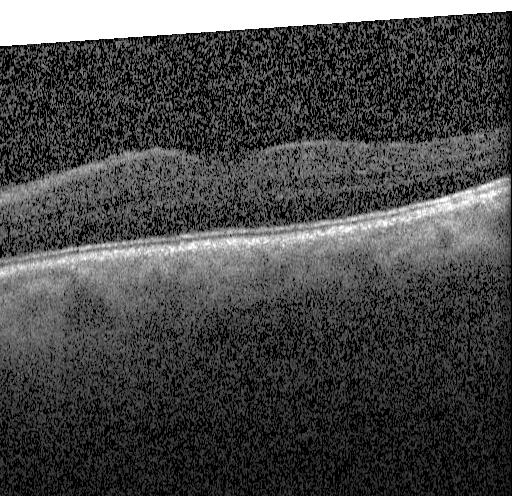 Optical coherence tomography B-scan; centered on the fovea. Macular OCT: no evidence of choroidal neovascularization, diabetic macular edema, or drusen.